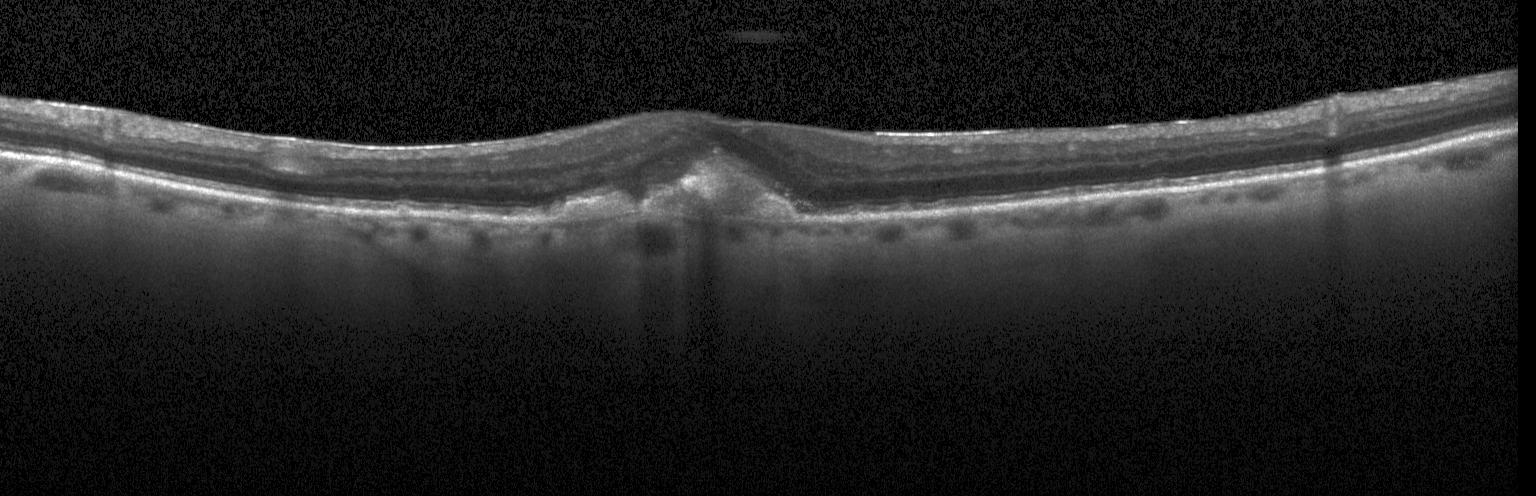
SD-OCT; optical coherence tomography B-scan; instrument: Heidelberg Spectralis; macular scan — This B-scan demonstrates a choroidal neovascular membrane.